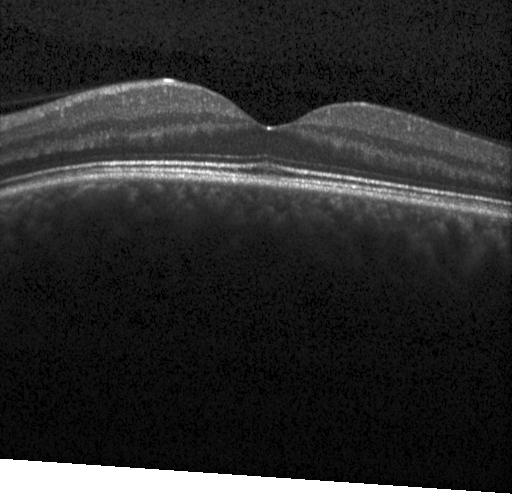
Horizontal scan through the fovea. Spectral-domain optical coherence tomography. OCT B-scan. The scan shows no choroidal neovascularization, diabetic macular edema, or drusen.